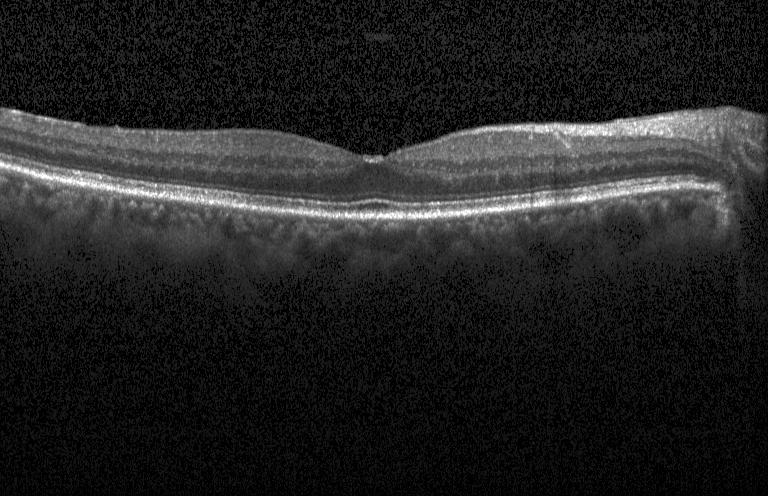
Optical coherence tomography scan.
Diagnosis: no choroidal neovascularization, diabetic macular edema, or drusen.